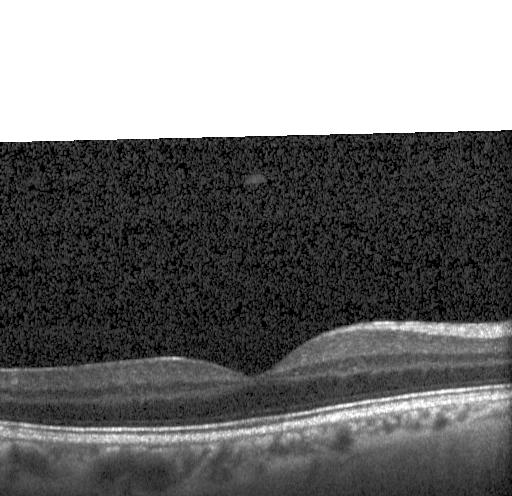

Macular OCT demonstrating no choroidal neovascularization, diabetic macular edema, or drusen.